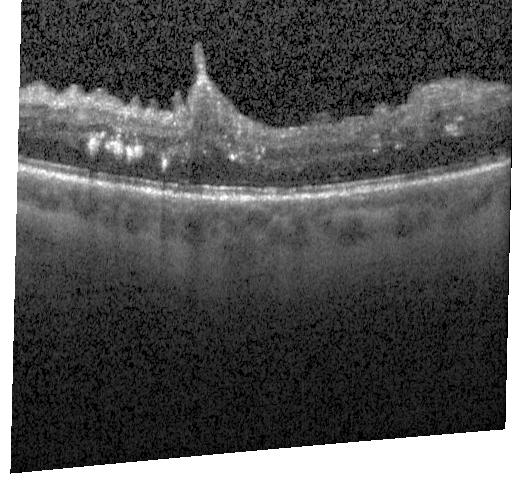
Macular scan; retinal OCT B-scan; Heidelberg Spectralis OCT system; spectral-domain optical coherence tomography
Diagnosis: diabetic macular edema.